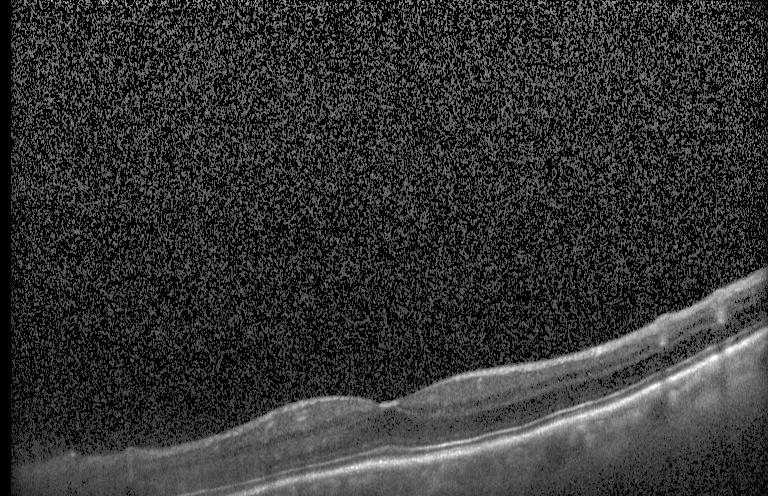

OCT B-scan showing neither CNV, DME, nor drusen.